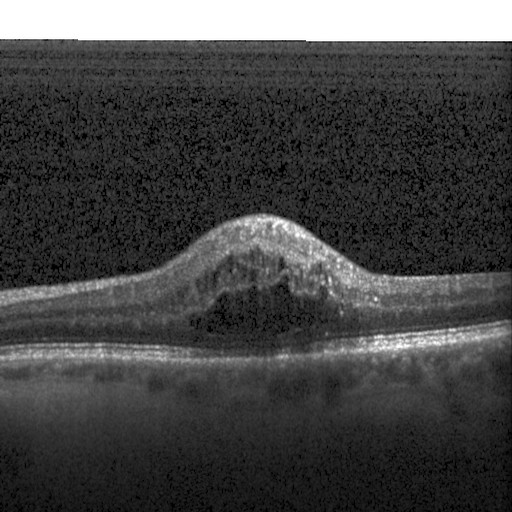 Assessment: DME.